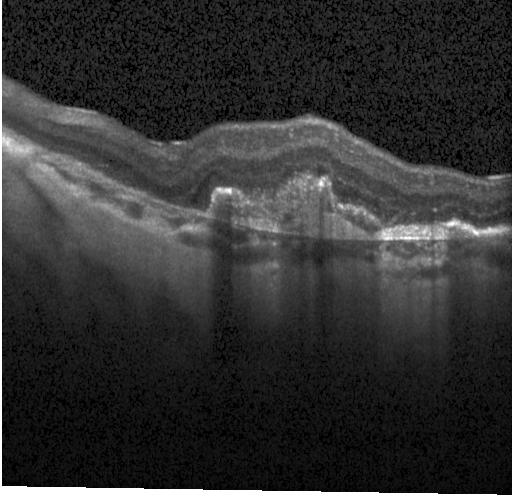

Optical coherence tomography scan
The scan shows a choroidal neovascular membrane.